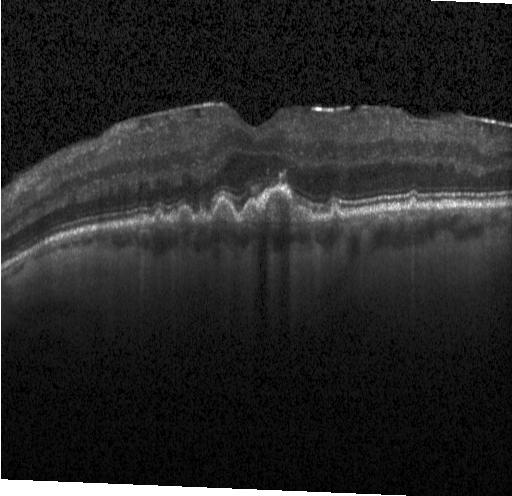
OCT line scan.
This B-scan demonstrates multiple drusen.